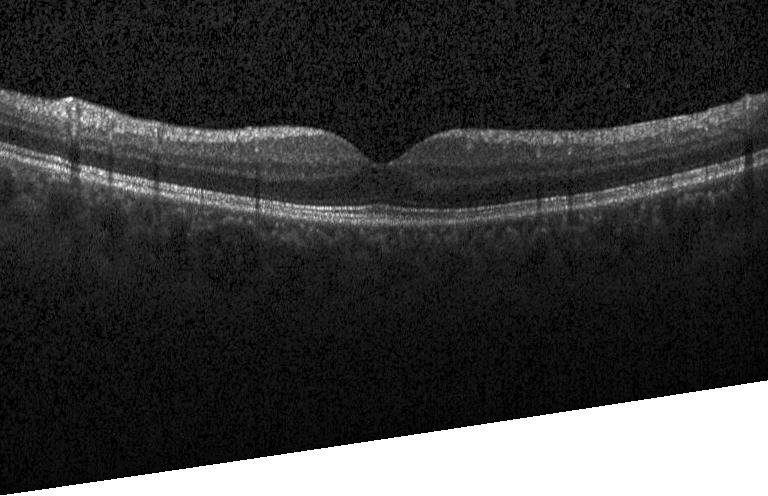

Acquired on a Heidelberg Spectralis; spectral-domain optical coherence tomography; OCT B-scan; fovea-centered
Impression: no choroidal neovascularization, diabetic macular edema, or drusen.